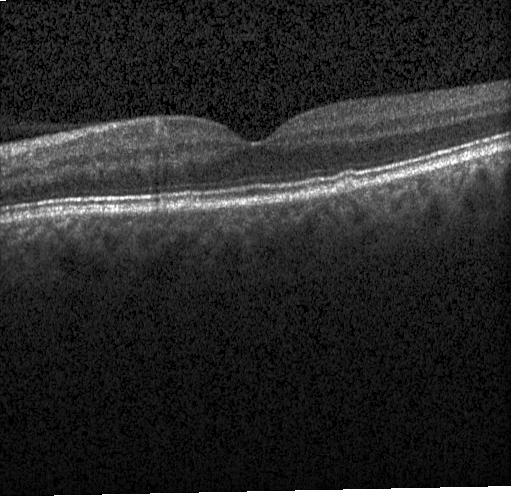

Acquired on a Heidelberg Spectralis · retinal OCT B-scan · spectral-domain optical coherence tomography · fovea-centered. Diagnosis: no choroidal neovascularization, diabetic macular edema, or drusen.